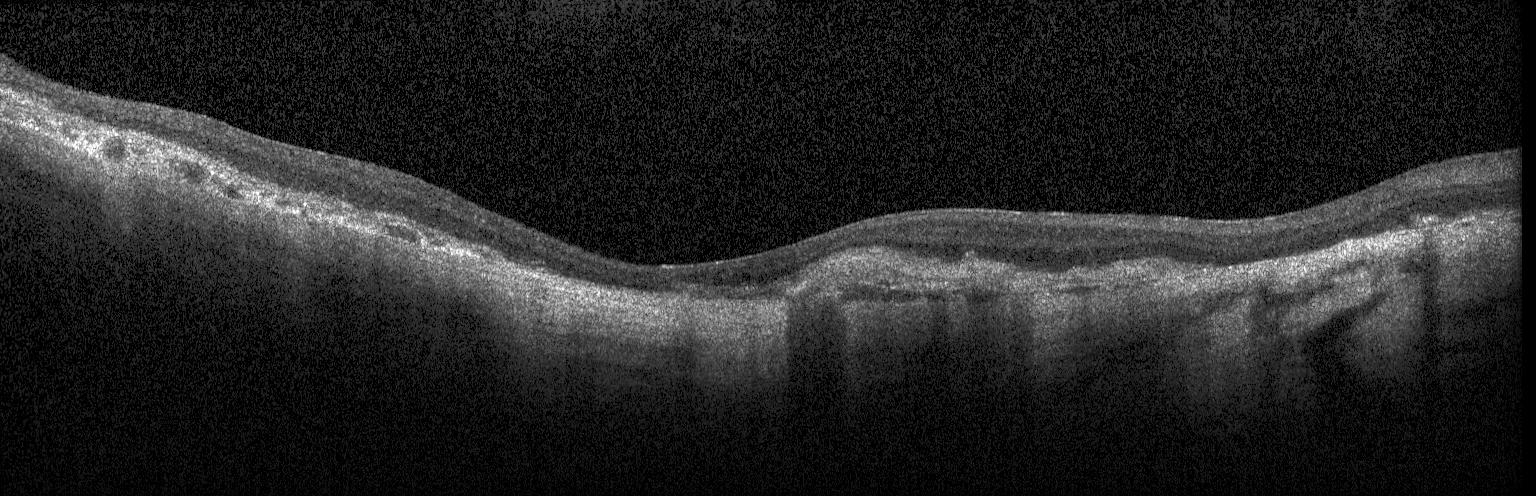 Spectral-domain OCT B-scan: CNV.